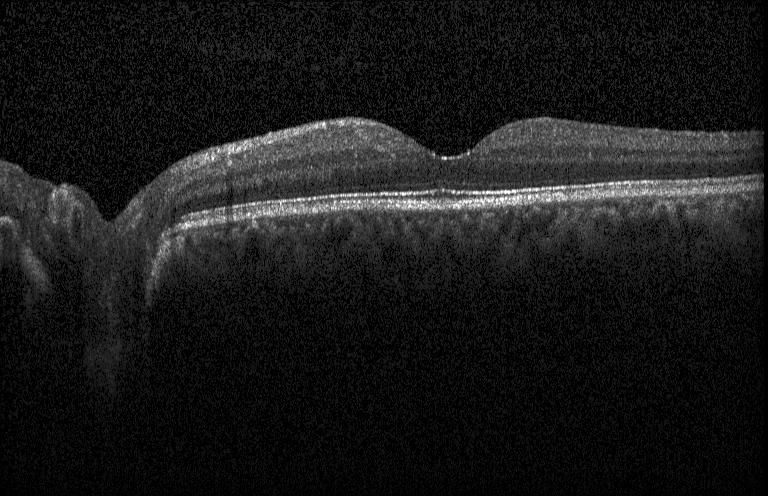

Finding: no choroidal neovascularization, no diabetic macular edema, and no drusen.